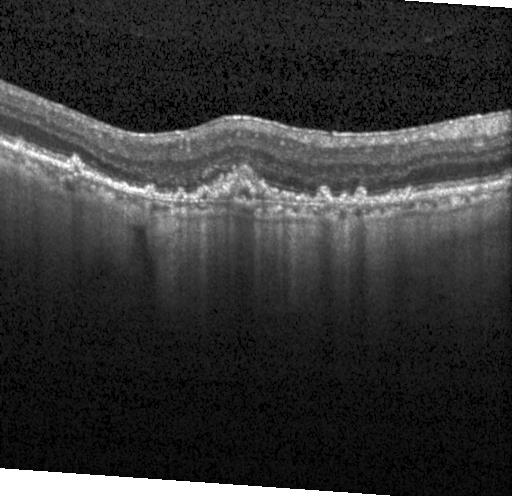
Diagnosis: a choroidal neovascular membrane.